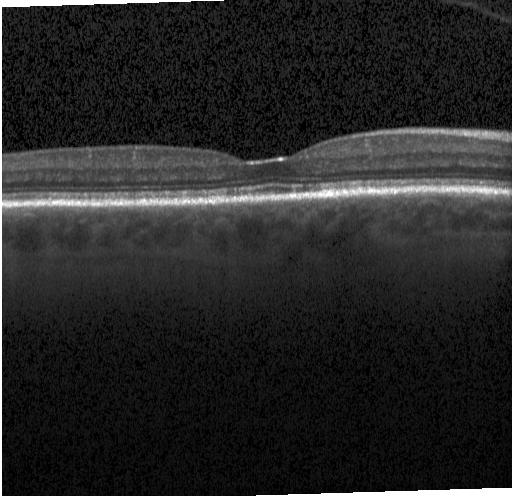
Diagnosis: no evidence of choroidal neovascularization, diabetic macular edema, or drusen.